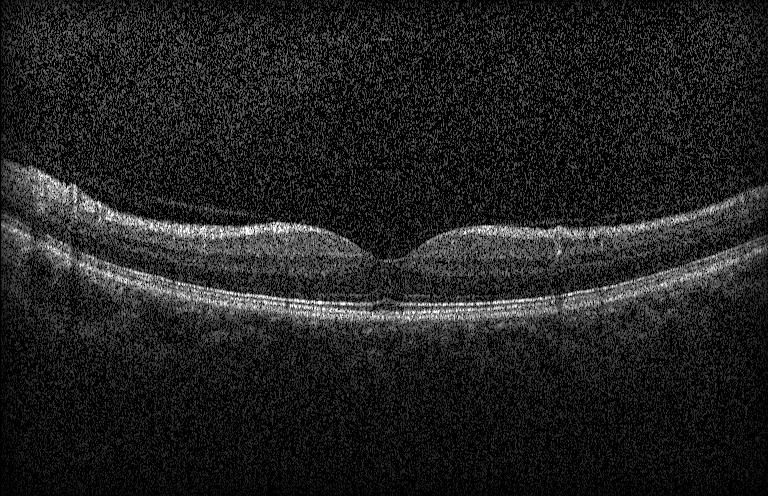

Horizontal scan through the fovea, spectral-domain optical coherence tomography, retinal OCT B-scan.
Finding: no CNV, no DME, and no drusen.